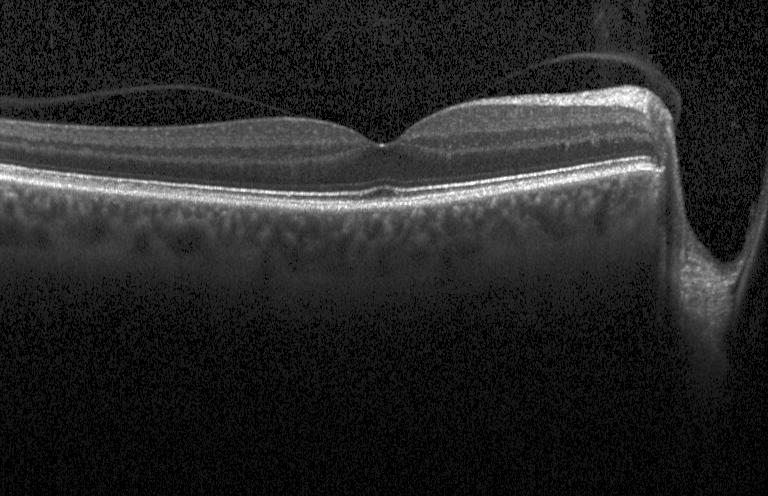 Instrument: Heidelberg Spectralis; OCT line scan; spectral-domain OCT. Impression: no choroidal neovascularization, no diabetic macular edema, and no drusen.